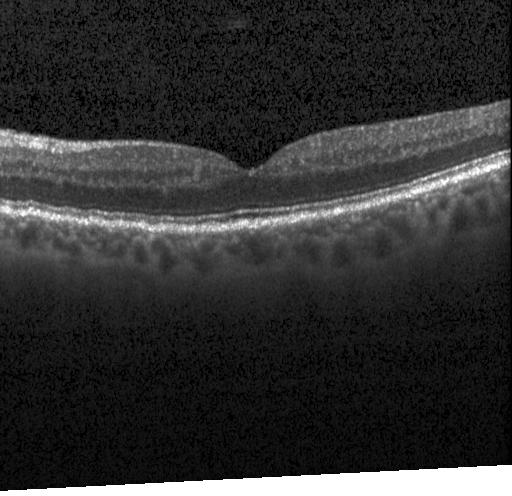
Diagnosis: no choroidal neovascularization, diabetic macular edema, or drusen.